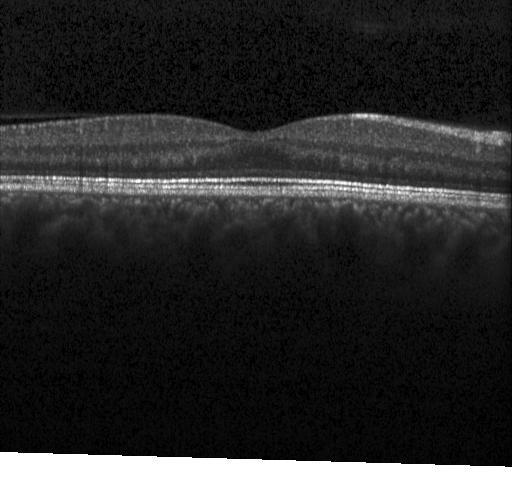

OCT line scan
Assessment: neither choroidal neovascularization, diabetic macular edema, nor drusen.